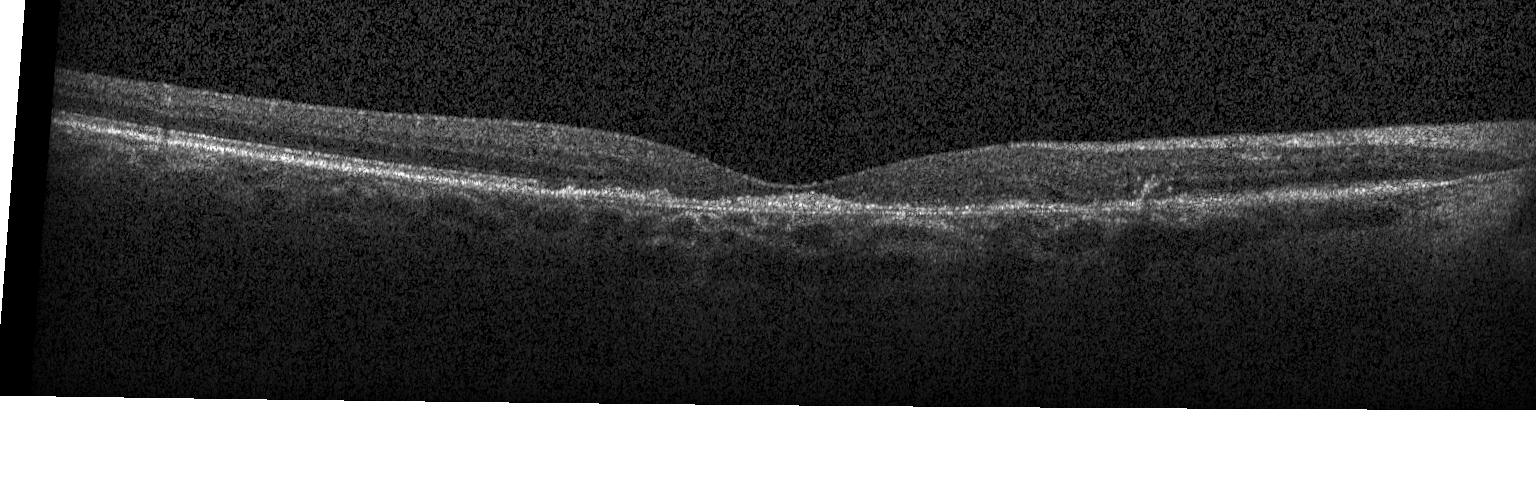
Impression: a choroidal neovascular membrane.